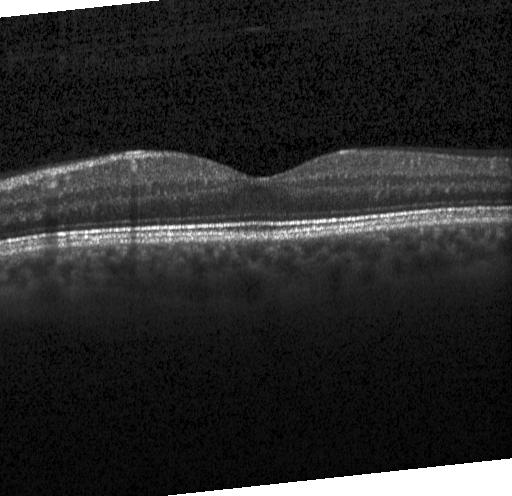

Centered on the fovea. Spectral-domain optical coherence tomography. Heidelberg Spectralis. OCT line scan — The scan shows no choroidal neovascularization, diabetic macular edema, or drusen.